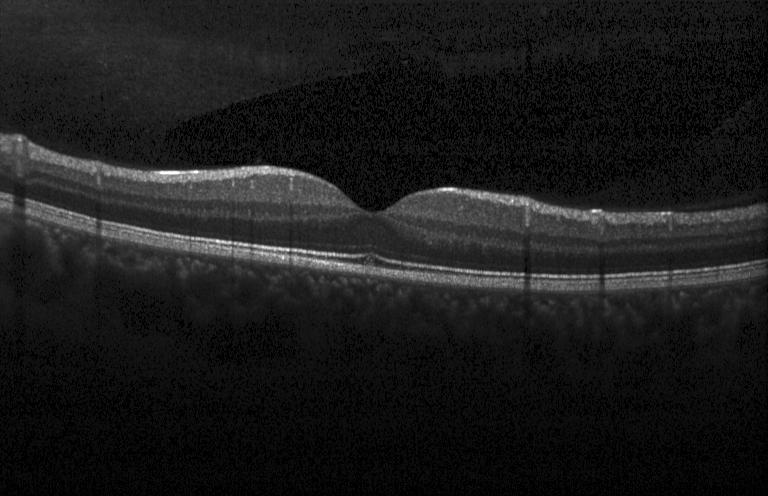
Diagnosis: no choroidal neovascularization, no diabetic macular edema, and no drusen.